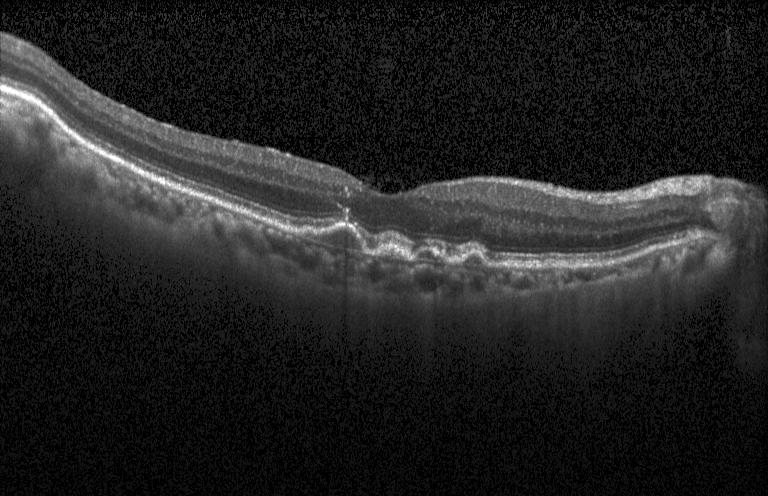 Retinal OCT B-scan
Finding: choroidal neovascularization.